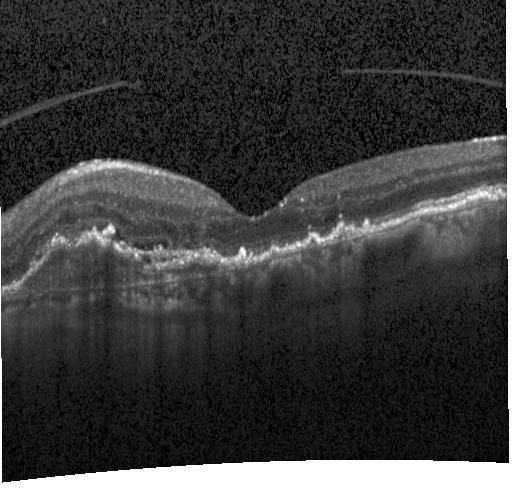 Instrument: Heidelberg Spectralis; centered on the fovea; retinal OCT cross-section; spectral-domain optical coherence tomography.
Diagnosis: choroidal neovascularization (CNV).